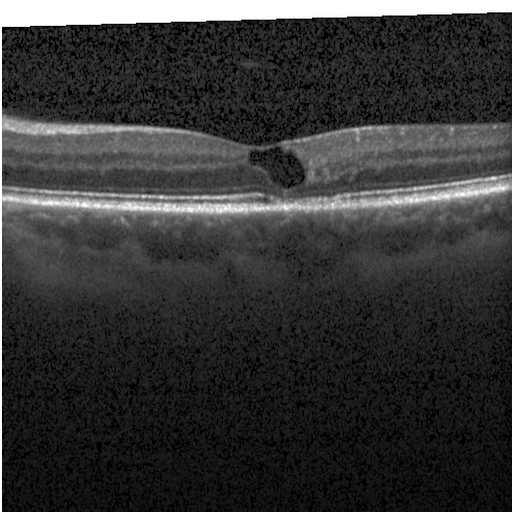

Heidelberg Spectralis · retinal OCT cross-section.
Finding: diabetic macular edema.